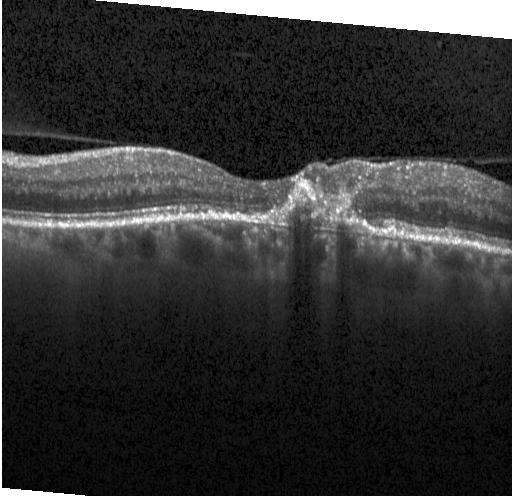

Optical coherence tomography scan. Impression: CNV.